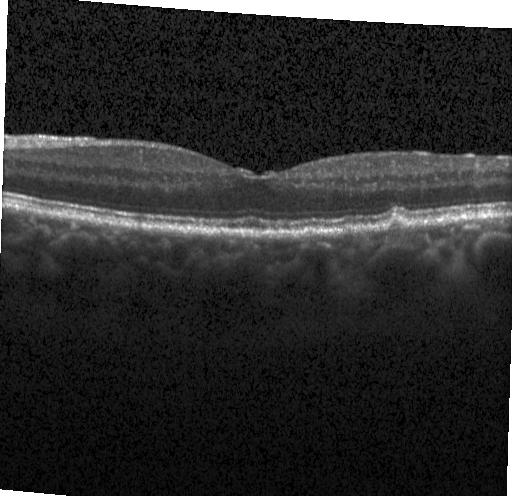

Finding: sub-RPE drusenoid deposits.